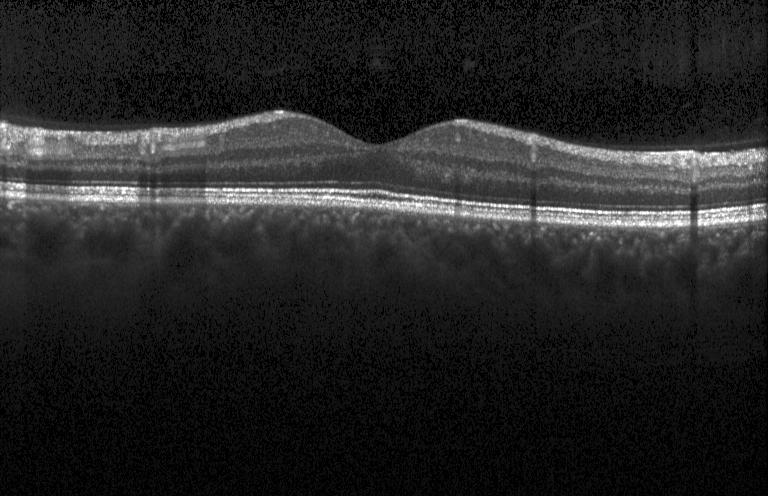

OCT finding: no choroidal neovascularization, no diabetic macular edema, and no drusen.